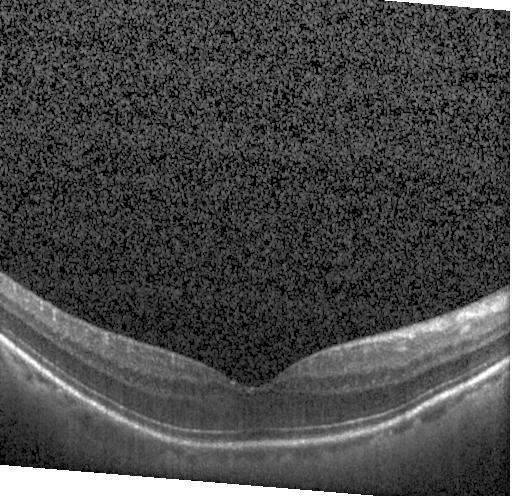

Diagnosis: no choroidal neovascularization, diabetic macular edema, or drusen.